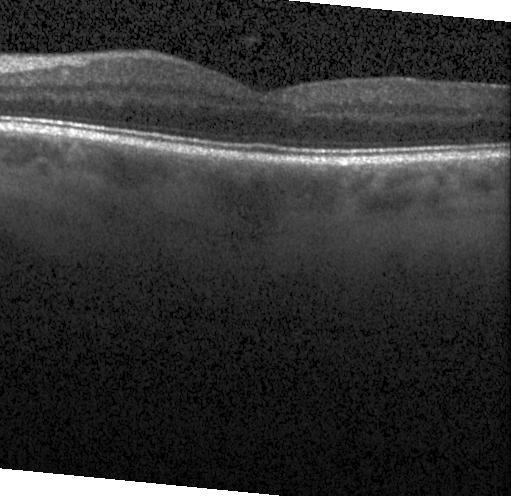

Retinal OCT cross-section, through the macula — Assessment: no CNV, no DME, and no drusen.